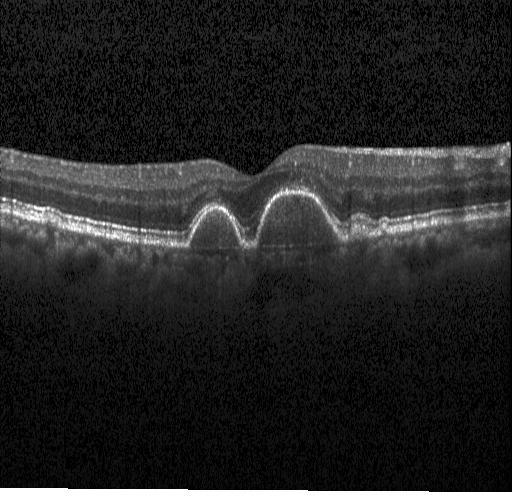

OCT line scan; spectral-domain OCT. Macular OCT: sub-RPE drusenoid deposits.